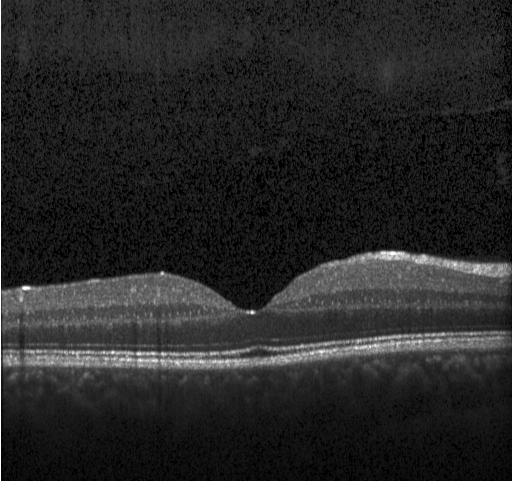
Retinal OCT cross-section. Centered on the fovea. Impression: no evidence of CNV, DME, or drusen.